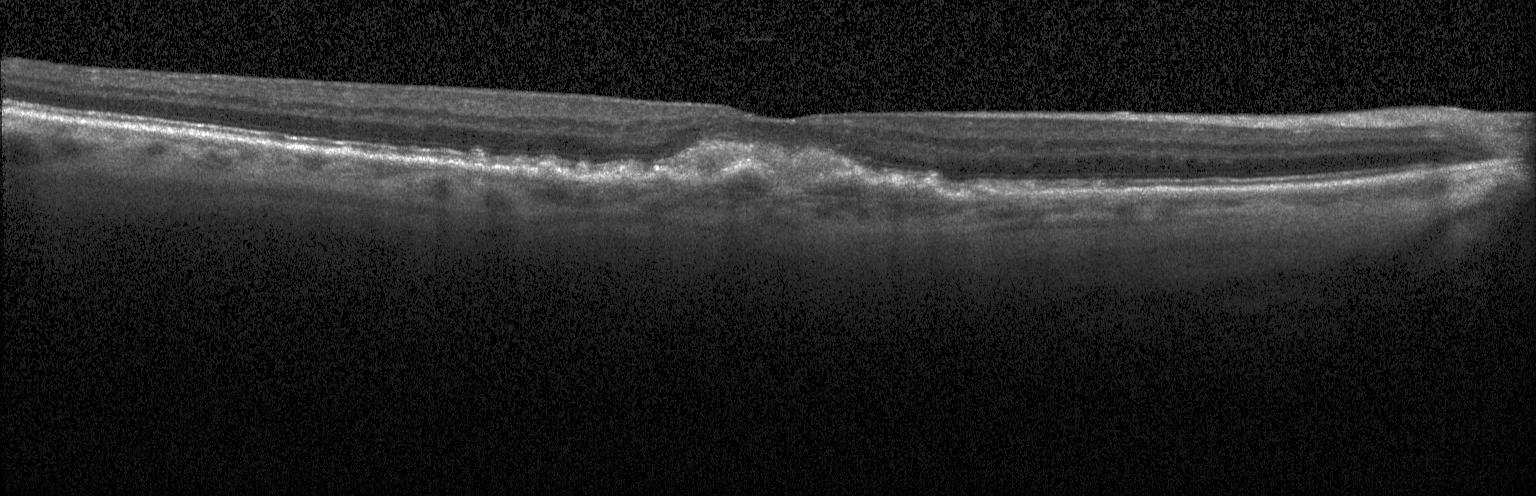

Spectral-domain OCT. Optical coherence tomography B-scan. Macular OCT: choroidal neovascularization (CNV).